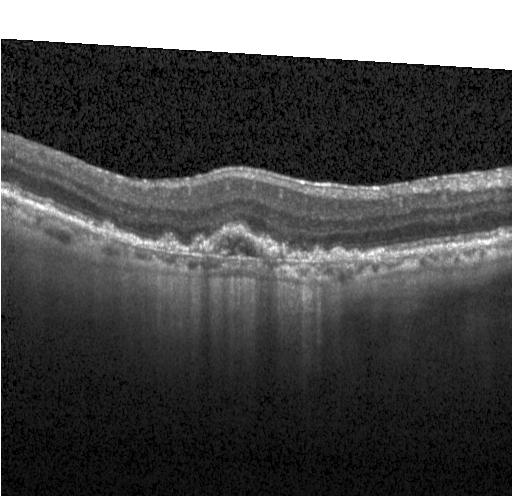

Macular OCT demonstrating choroidal neovascularization.